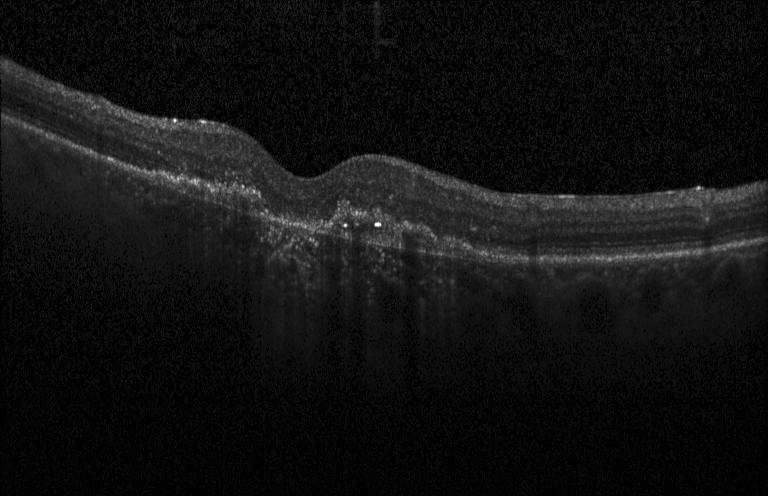
OCT B-scan, Heidelberg Spectralis OCT system. Diagnosis: a choroidal neovascular membrane.